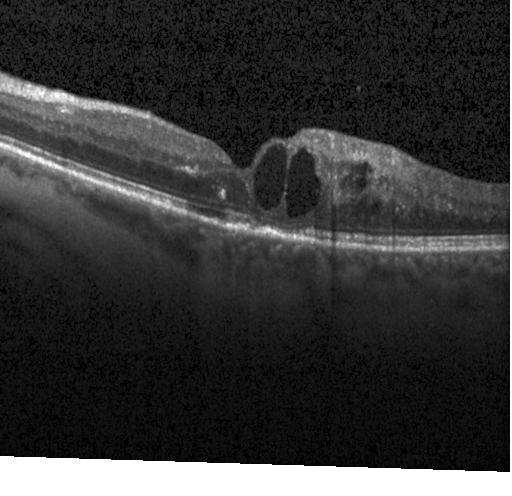
Macular OCT: diabetic macular edema (DME).